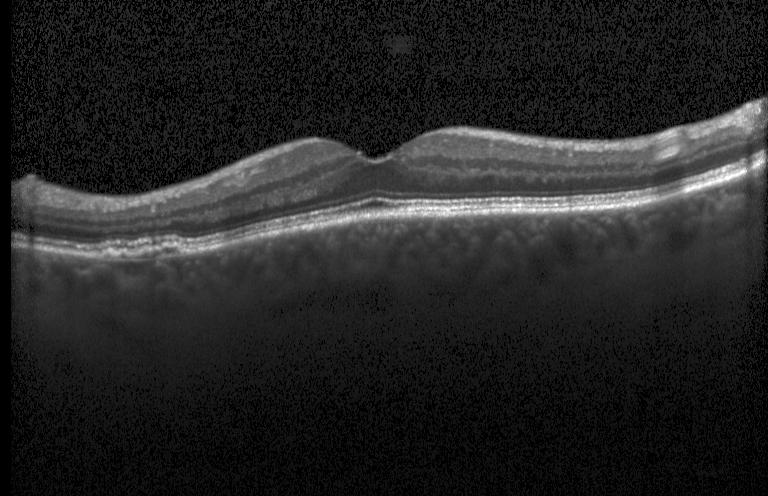
Macular OCT: a choroidal neovascular membrane.